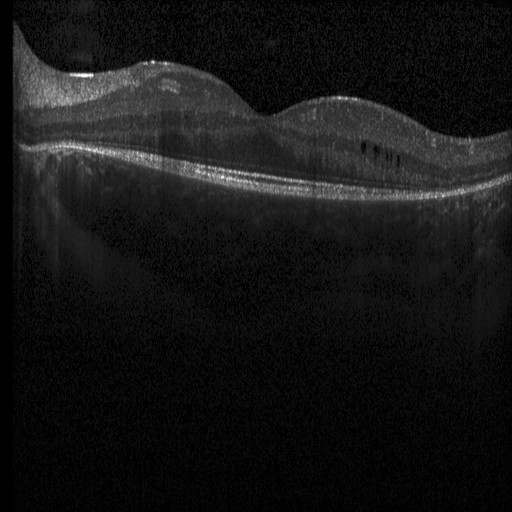

OCT line scan. Finding: diabetic macular edema (DME).